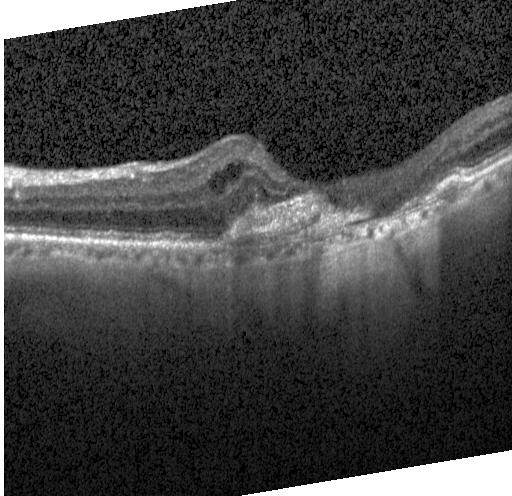

Macular scan, retinal OCT cross-section. Impression: a choroidal neovascular membrane.